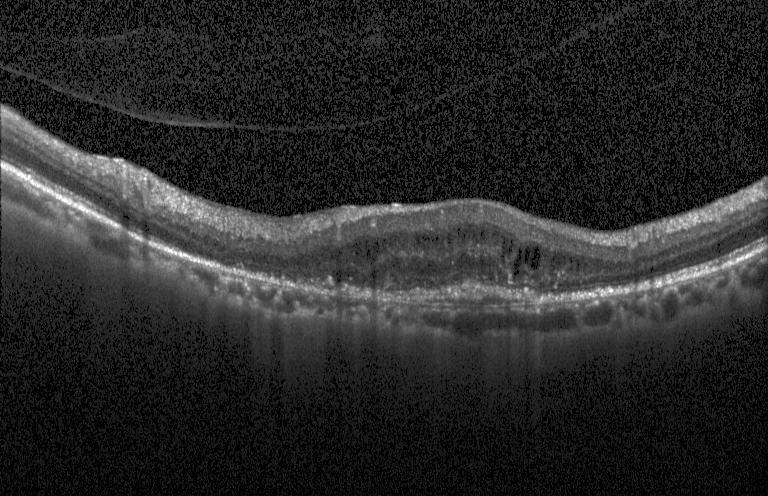
Finding: choroidal neovascularization (CNV).